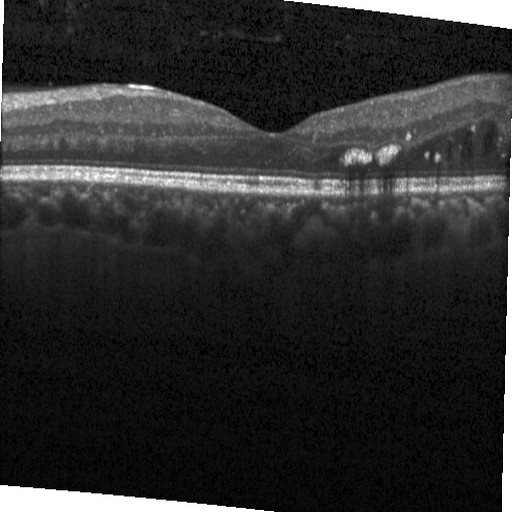 Retinal OCT cross-section · acquired on a Heidelberg Spectralis · through the macula.
Impression: diabetic macular edema.